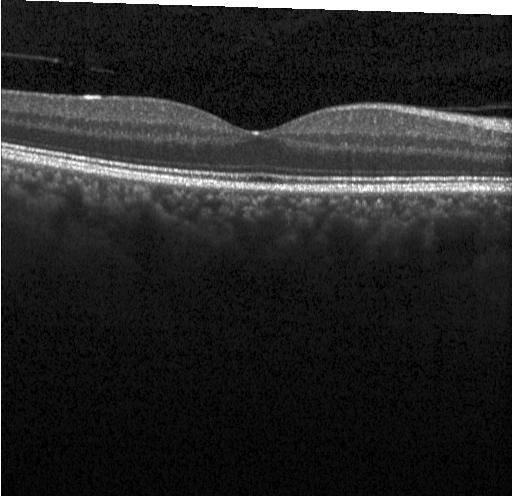
Heidelberg Spectralis, retinal OCT cross-section.
OCT finding: no choroidal neovascularization, diabetic macular edema, or drusen.